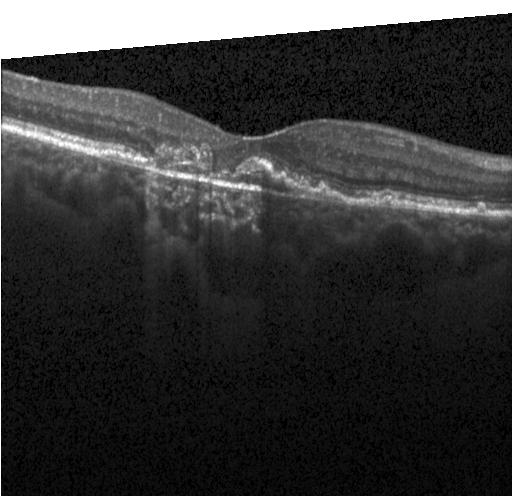

OCT line scan
Impression: a choroidal neovascular membrane.